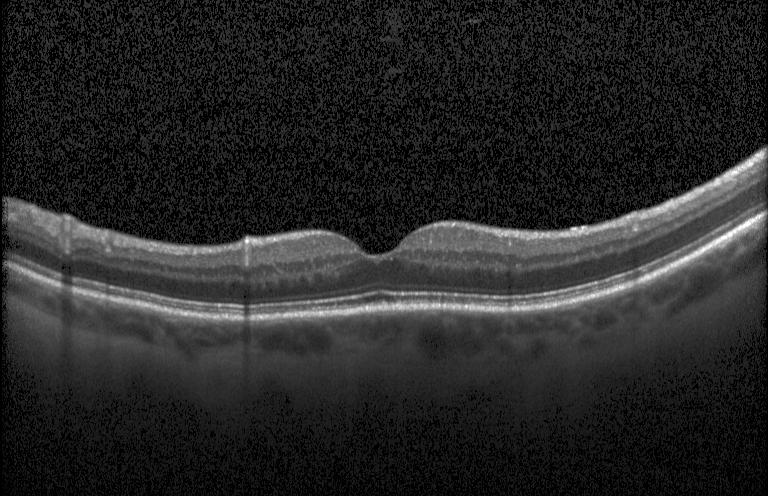
Acquired on a Heidelberg Spectralis · retinal OCT B-scan — Diagnosis: no choroidal neovascularization, diabetic macular edema, or drusen.